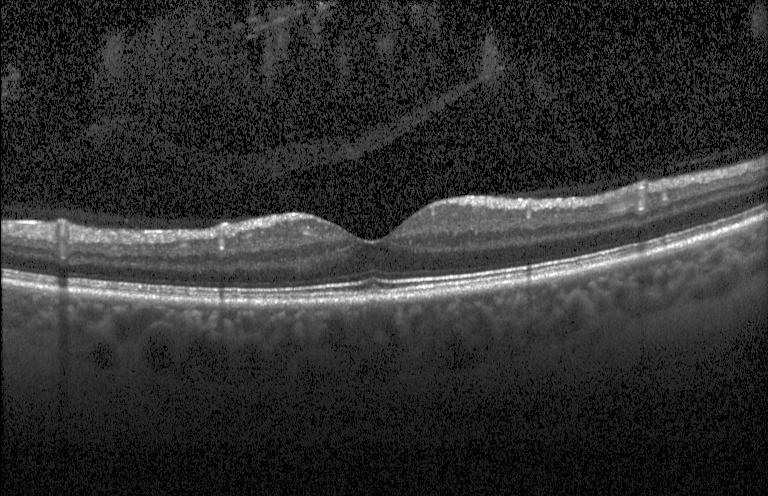 SD-OCT · instrument: Heidelberg Spectralis · centered on the fovea · optical coherence tomography B-scan — The scan shows neither choroidal neovascularization, diabetic macular edema, nor drusen.